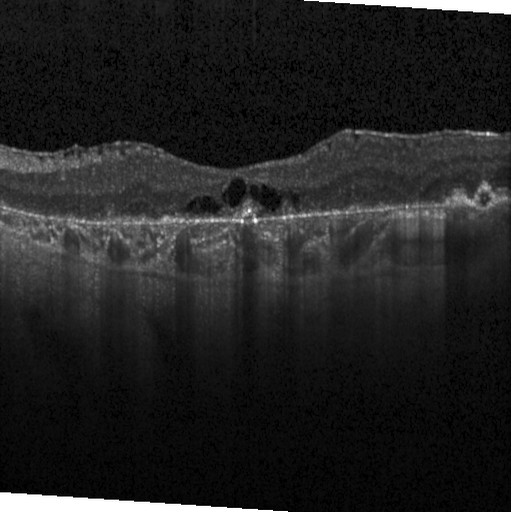

Diabetic macular edema (DME).